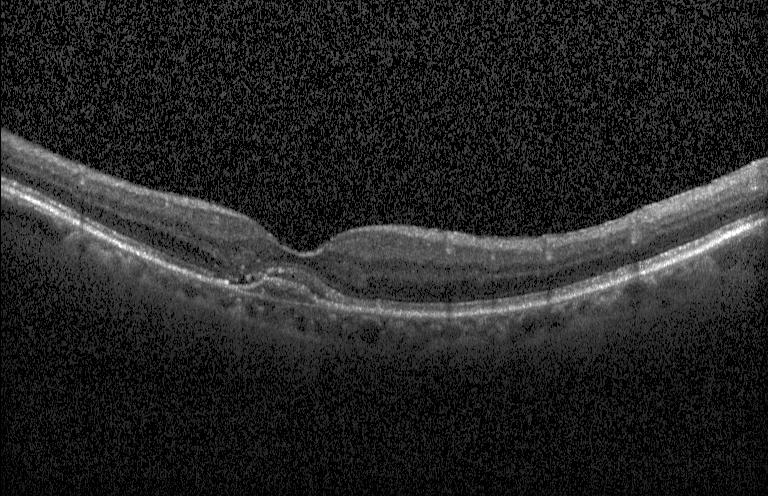 Retinal OCT cross-section showing choroidal neovascularization.